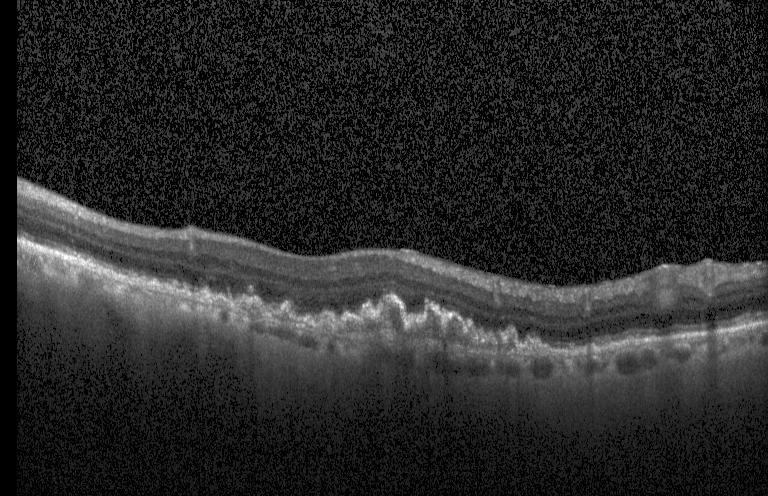
OCT B-scan showing a choroidal neovascular membrane.